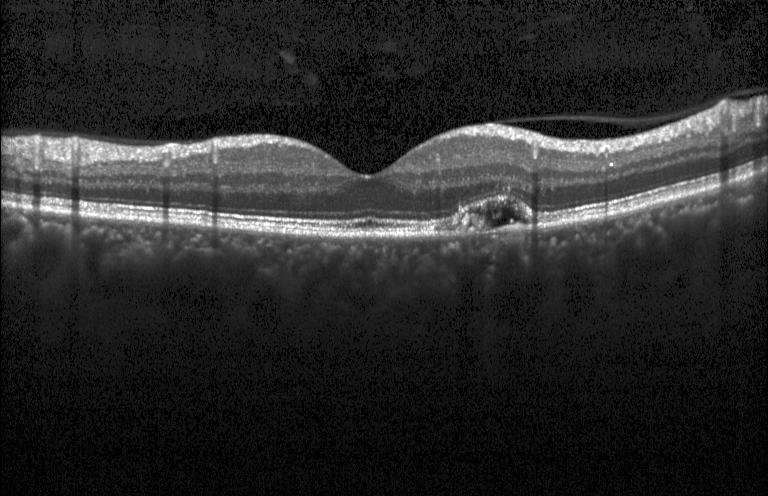

A choroidal neovascular membrane.